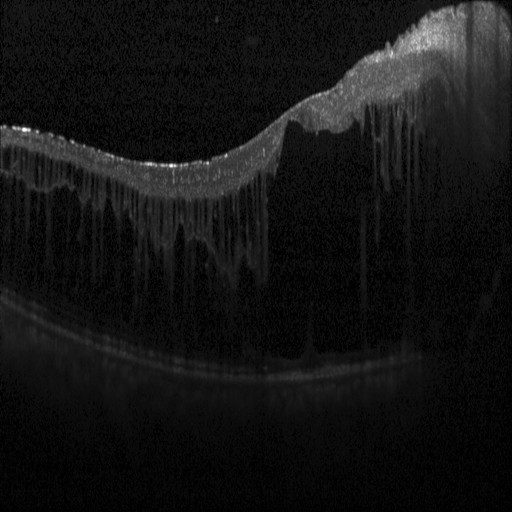

Through the macula · SD-OCT · retinal OCT B-scan · instrument: Heidelberg Spectralis
Finding: diabetic macular edema (DME).